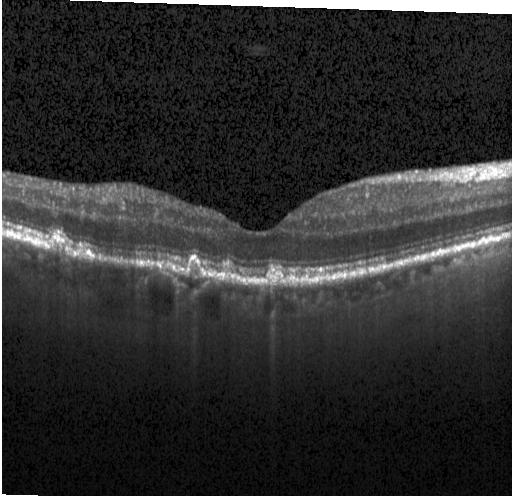 Optical coherence tomography B-scan. Impression: multiple drusen.